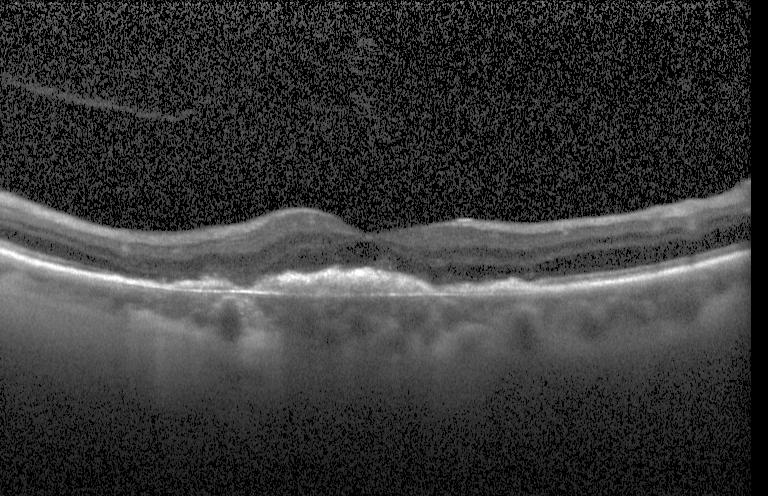

Spectral-domain OCT B-scan: a choroidal neovascular membrane.